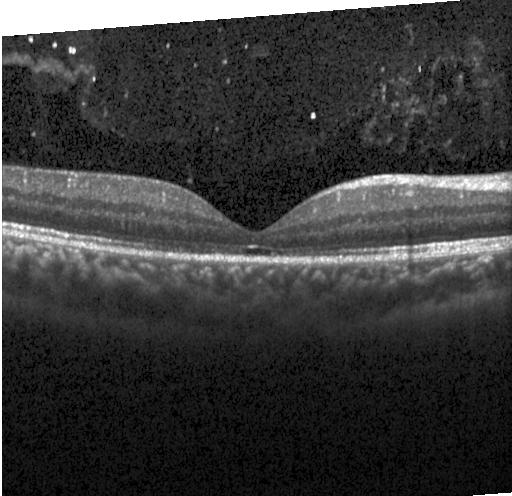

Diagnosis: neither CNV, DME, nor drusen.